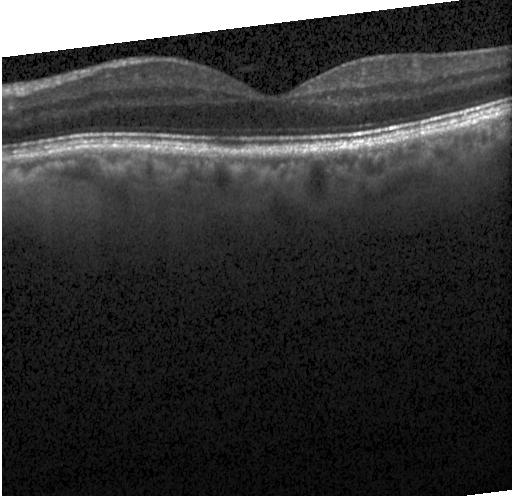

Fovea-centered, retinal OCT B-scan, instrument: Heidelberg Spectralis, spectral-domain optical coherence tomography.
Diagnosis: neither choroidal neovascularization, diabetic macular edema, nor drusen.